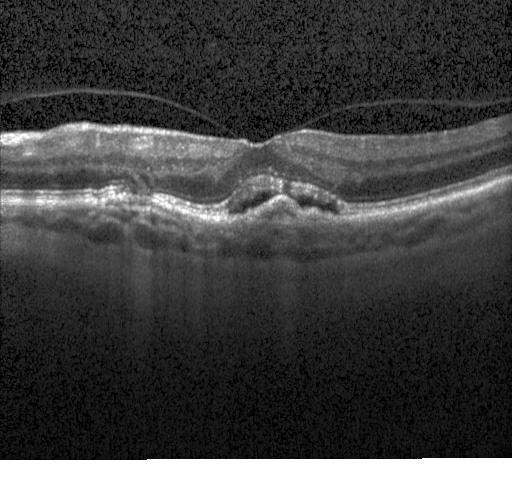
Impression: a choroidal neovascular membrane.